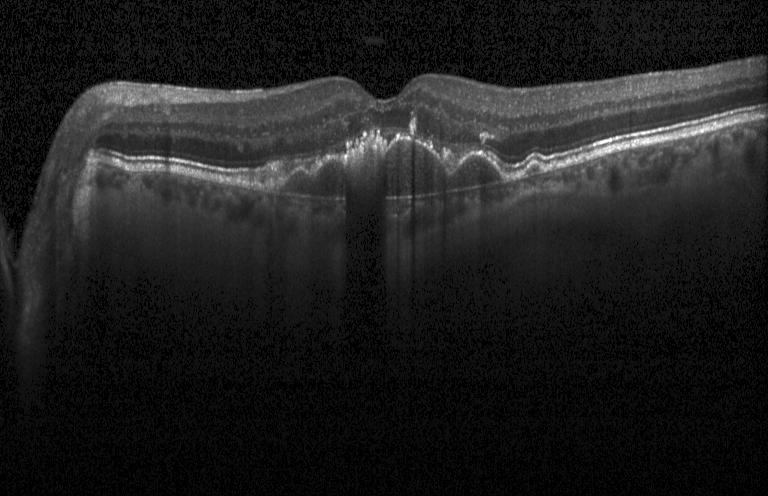 OCT finding: a choroidal neovascular membrane.